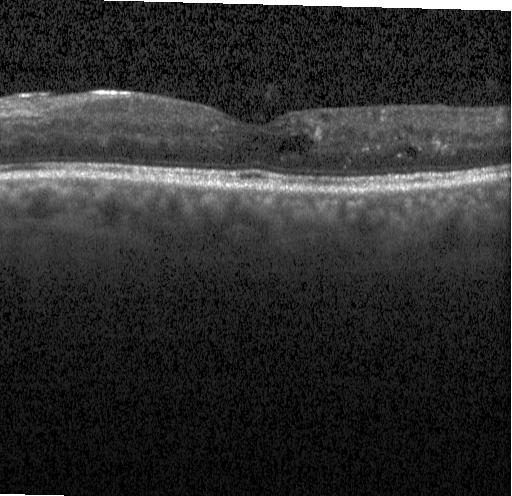
Optical coherence tomography scan — Assessment: diabetic macular edema (DME).